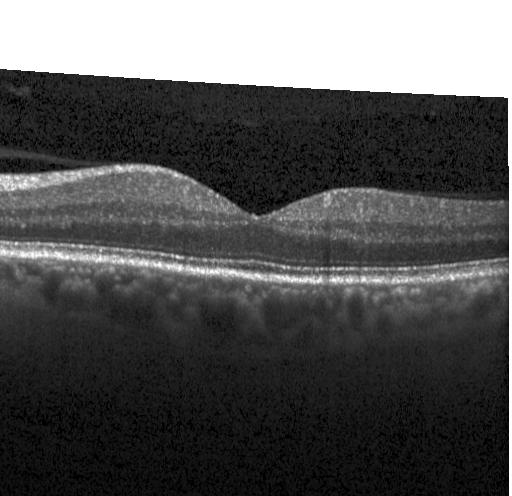
Heidelberg Spectralis OCT system; centered on the fovea; OCT B-scan; spectral-domain OCT — Assessment: no choroidal neovascularization, no diabetic macular edema, and no drusen.